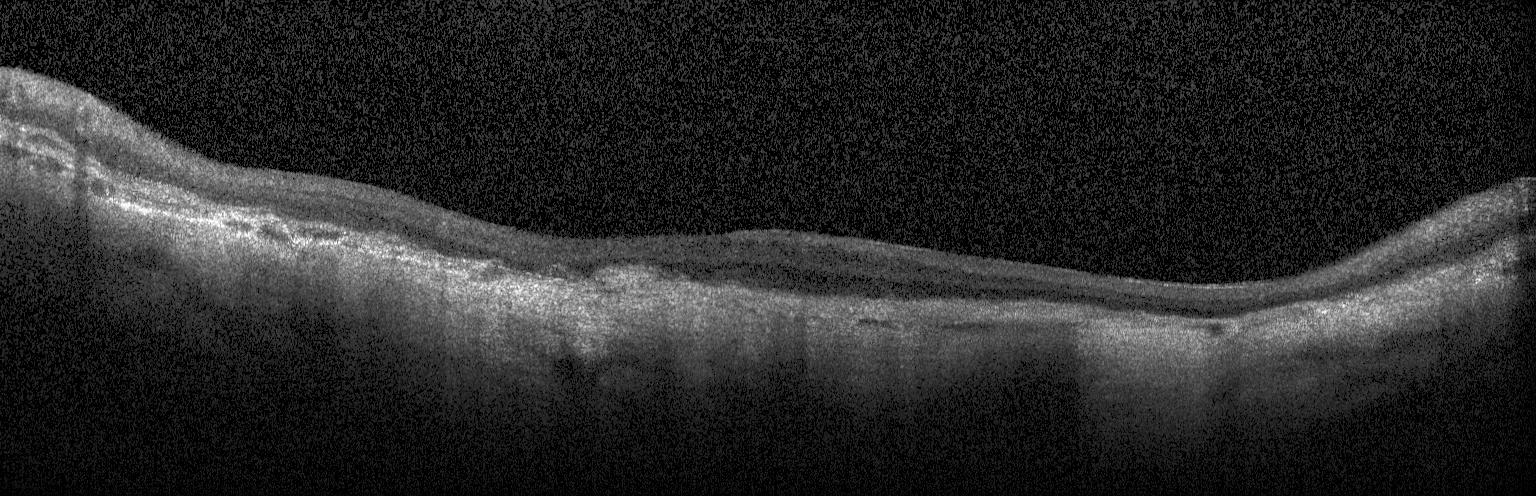
Acquired on a Heidelberg Spectralis · SD-OCT · macular scan · retinal OCT B-scan.
OCT finding: choroidal neovascularization (CNV).